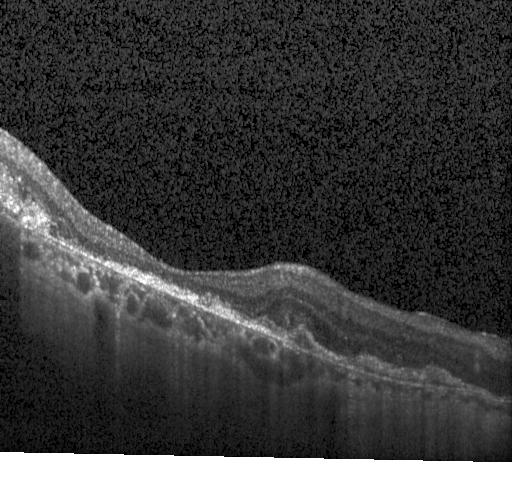
SD-OCT, macular scan, optical coherence tomography scan — Impression: a choroidal neovascular membrane.